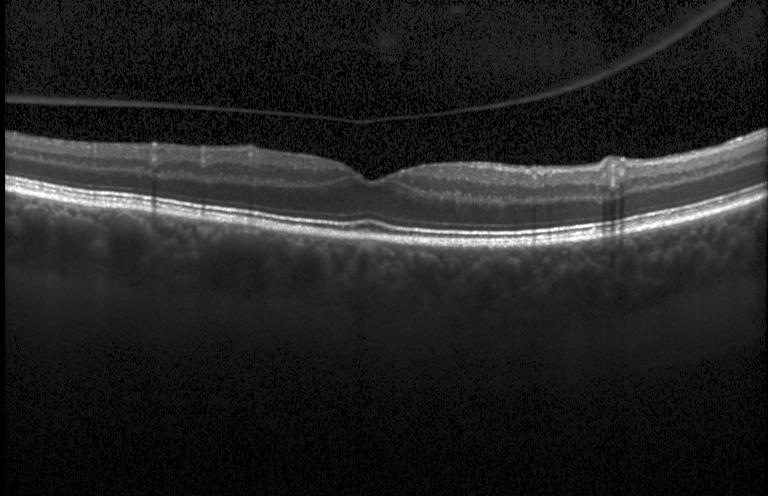 Through the macula · optical coherence tomography scan. Diagnosis: no CNV, DME, or drusen.